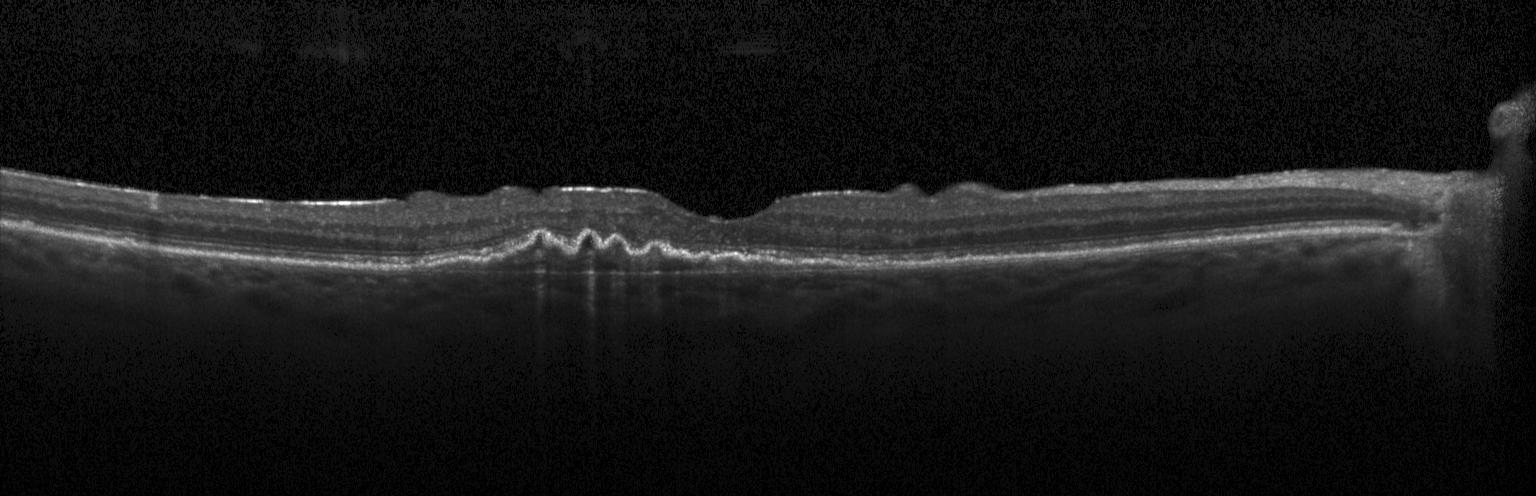
OCT finding: choroidal neovascularization.